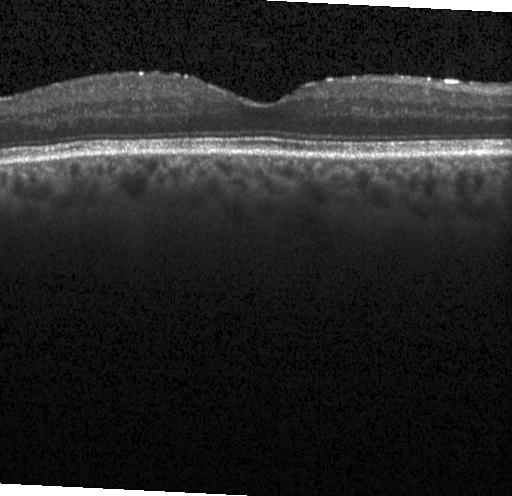 Retinal OCT B-scan; spectral-domain optical coherence tomography; through the macula
Impression: neither choroidal neovascularization, diabetic macular edema, nor drusen.